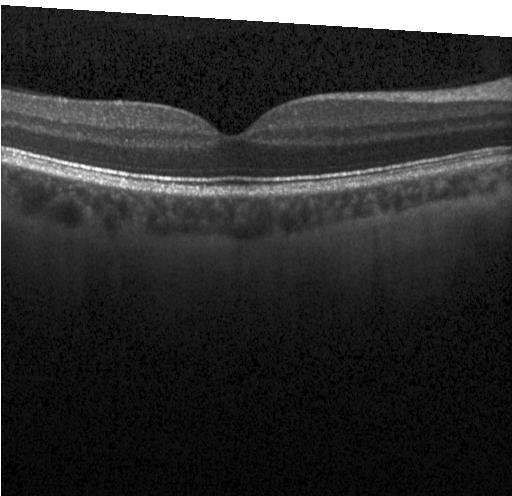

No choroidal neovascularization, no diabetic macular edema, and no drusen.